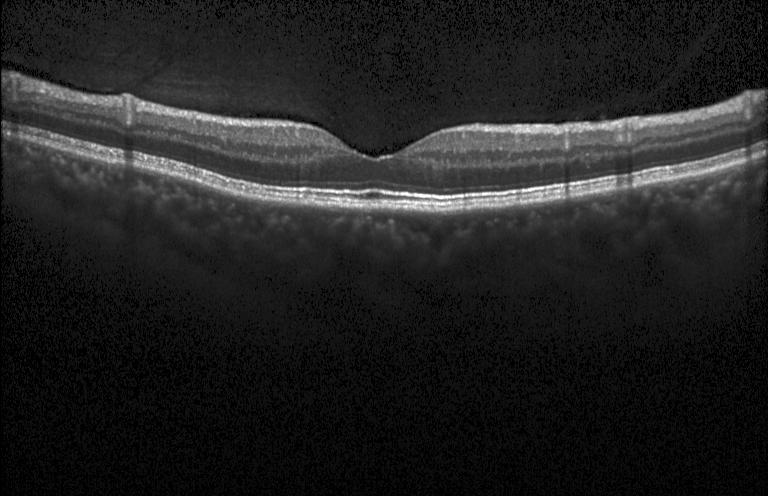

Spectral-domain optical coherence tomography, Heidelberg Spectralis OCT system, retinal OCT cross-section, fovea-centered — Macular OCT: neither choroidal neovascularization, diabetic macular edema, nor drusen.